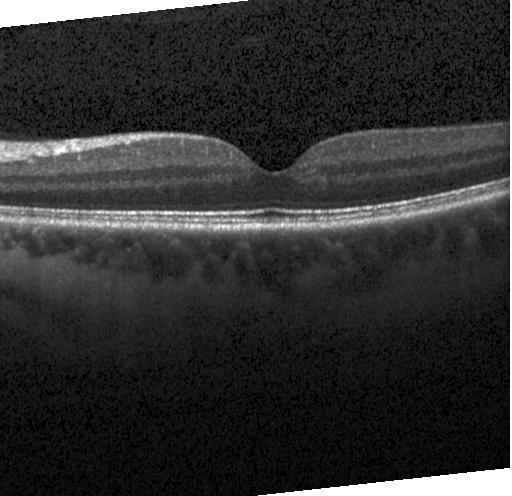 This B-scan demonstrates no CNV, DME, or drusen.